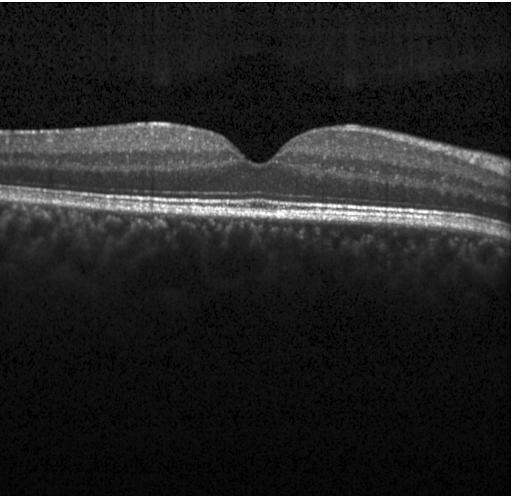
Retinal OCT cross-section showing no choroidal neovascularization, diabetic macular edema, or drusen.